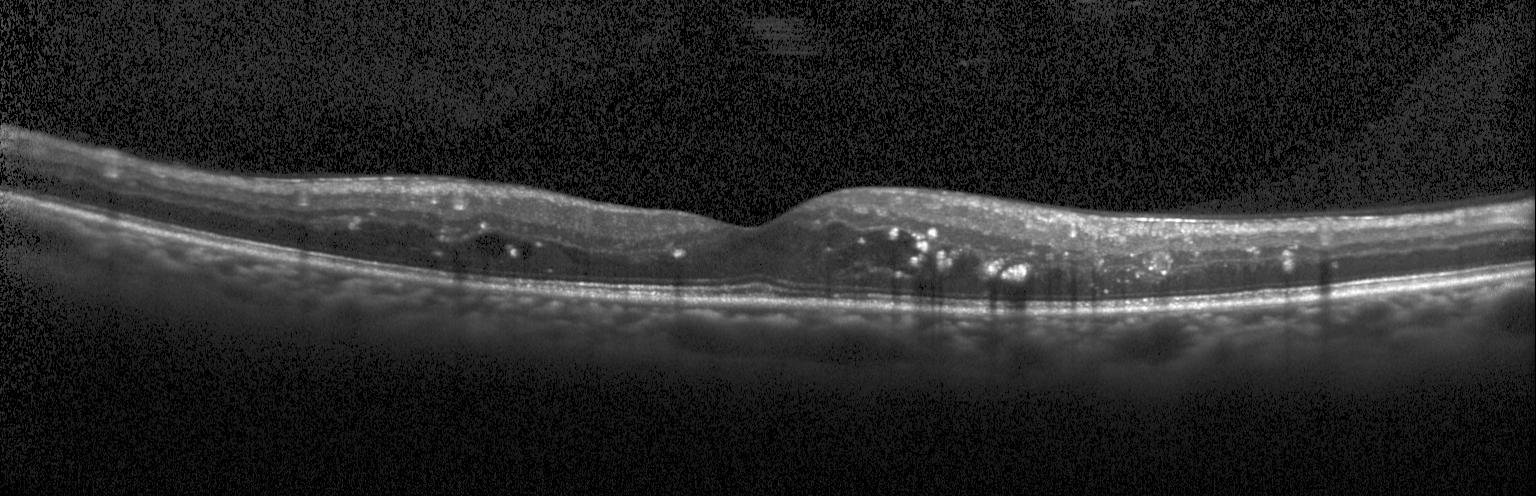 Spectral-domain OCT B-scan: DME.